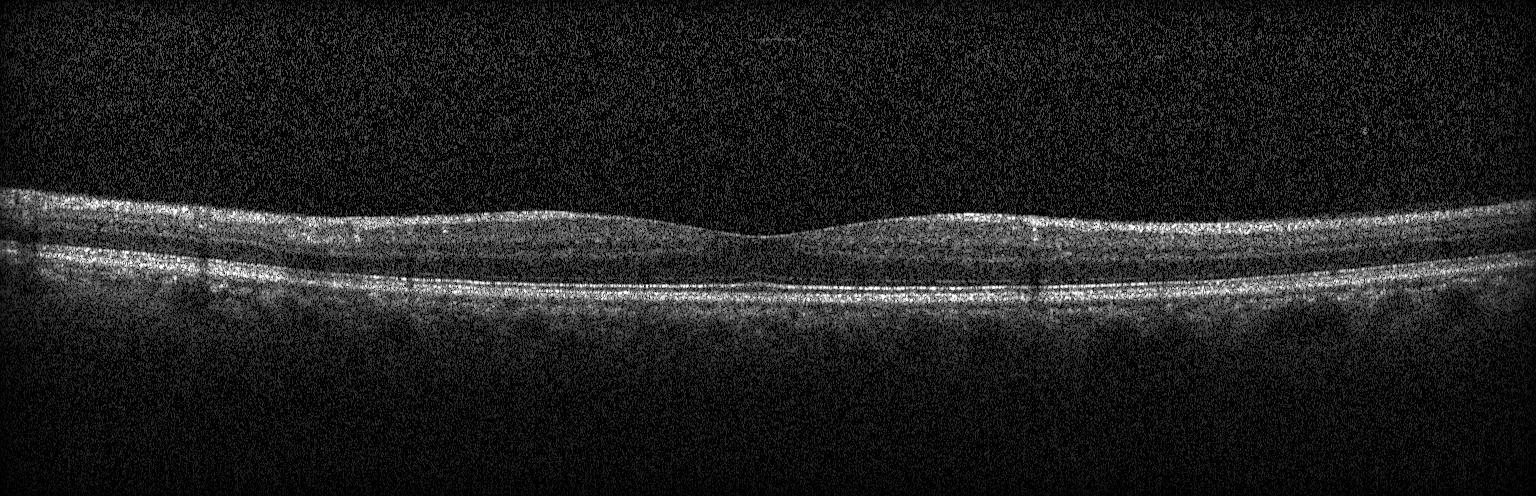 Spectral-domain OCT · through the macula · retinal OCT B-scan · Heidelberg Spectralis OCT system — Diagnosis: no choroidal neovascularization, no diabetic macular edema, and no drusen.